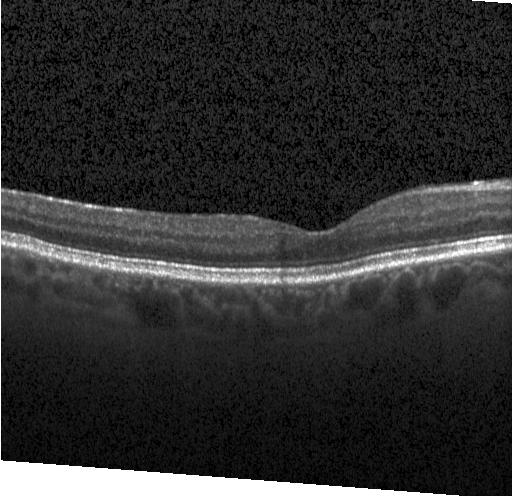

OCT B-scan · through the macula · spectral-domain optical coherence tomography — Finding: no evidence of choroidal neovascularization, diabetic macular edema, or drusen.